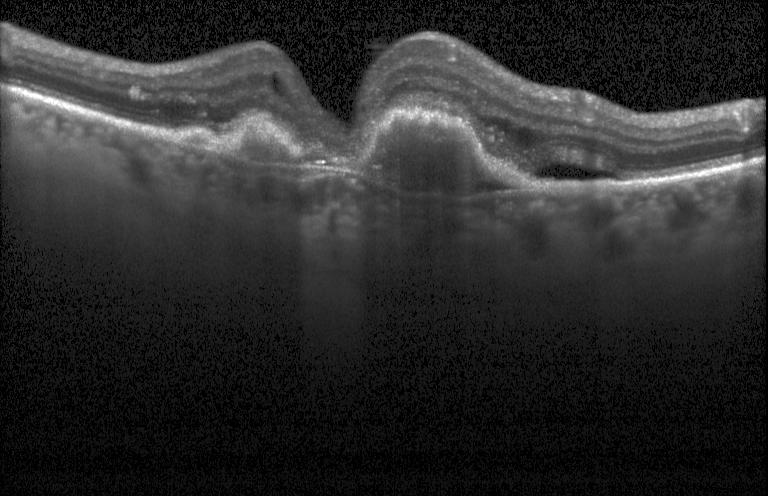 Dx: choroidal neovascularization (CNV).